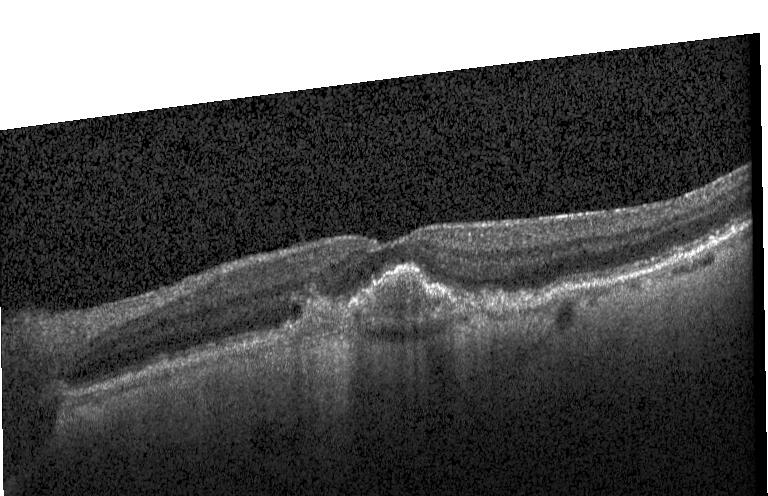 Macular OCT demonstrating choroidal neovascularization.